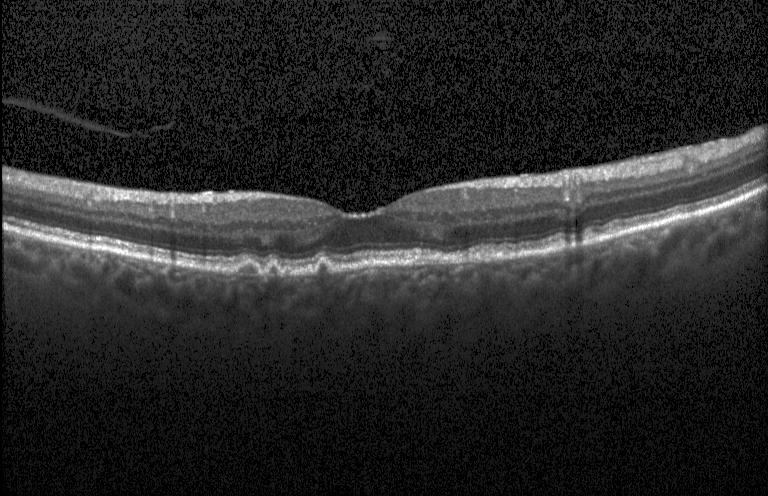
Retinal OCT cross-section showing drusen.